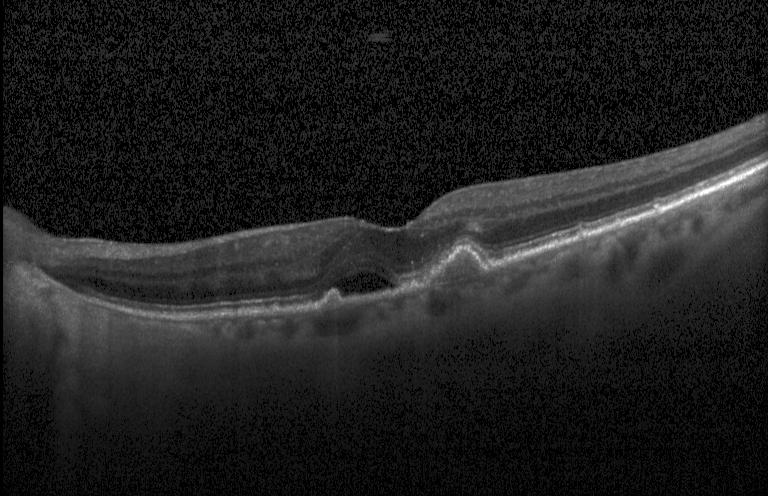

Instrument: Heidelberg Spectralis; optical coherence tomography scan — This B-scan demonstrates choroidal neovascularization (CNV).